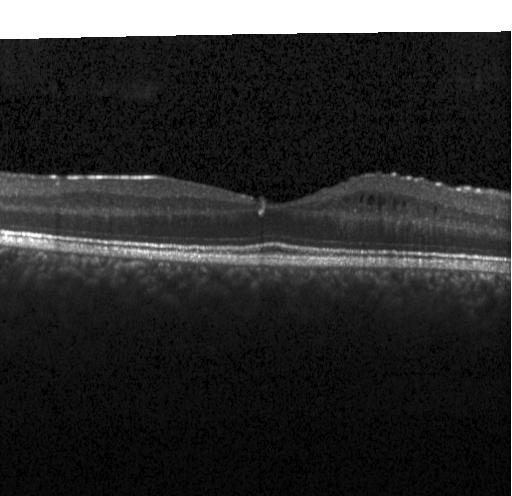 Dx: DME.